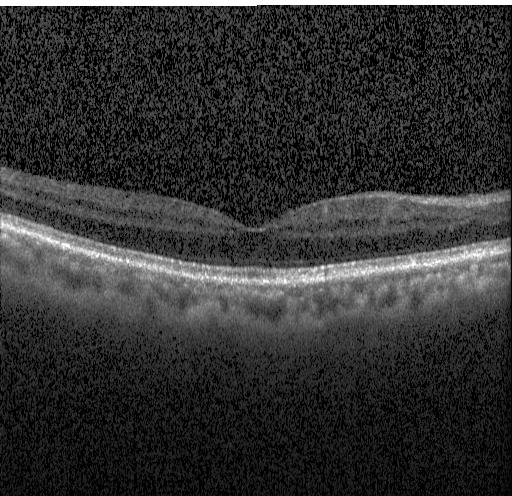 OCT B-scan; Heidelberg Spectralis OCT system; spectral-domain optical coherence tomography. The scan shows no CNV, no DME, and no drusen.